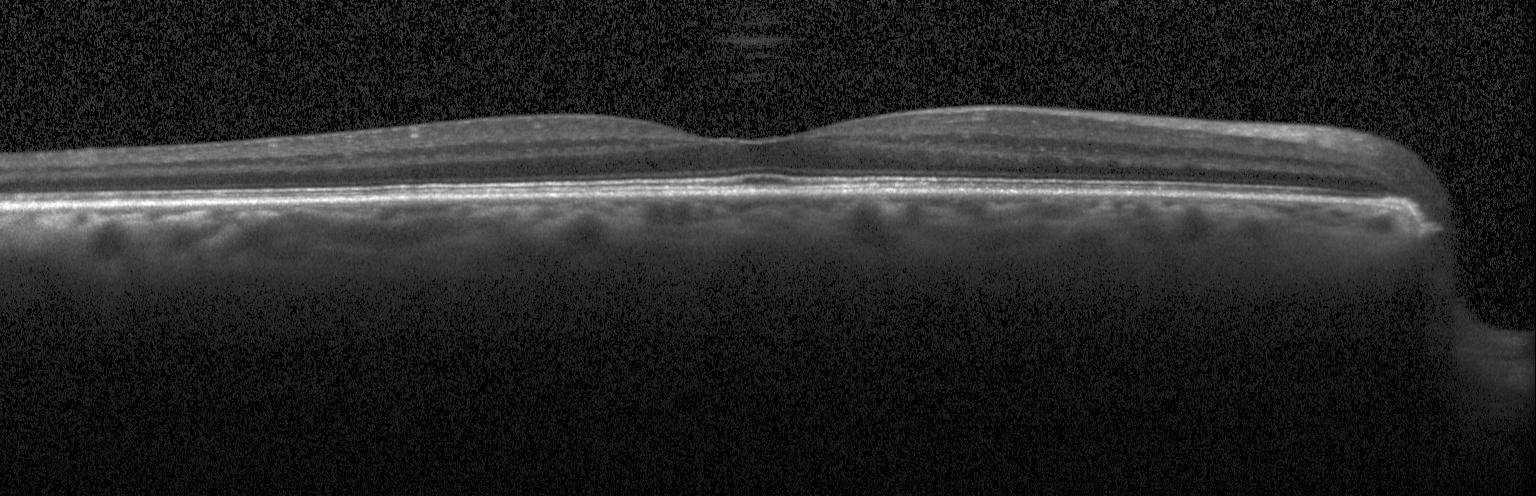 Assessment: no choroidal neovascularization, diabetic macular edema, or drusen.